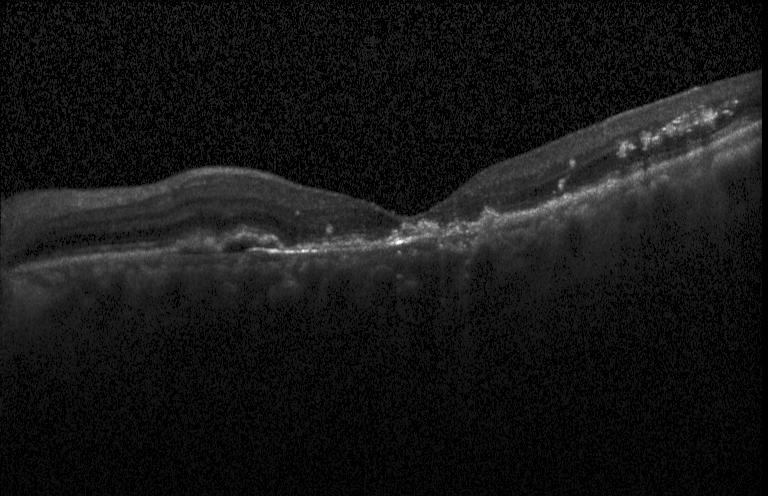

Acquired on a Heidelberg Spectralis; horizontal scan through the fovea; optical coherence tomography B-scan.
Dx: choroidal neovascularization.